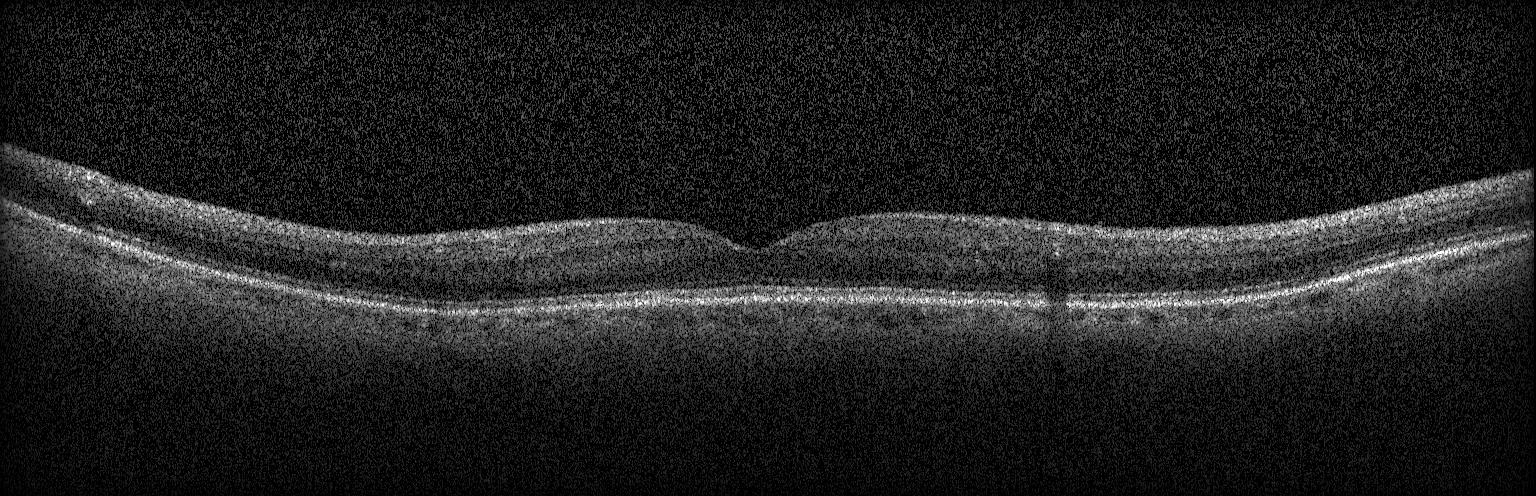 Acquired on a Heidelberg Spectralis. Retinal OCT cross-section — The scan shows no choroidal neovascularization, no diabetic macular edema, and no drusen.